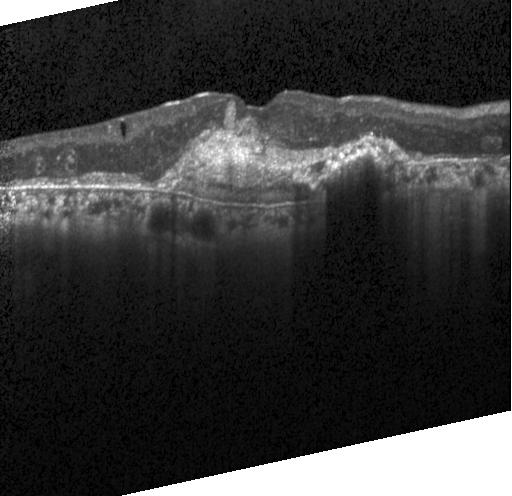

OCT finding: CNV.